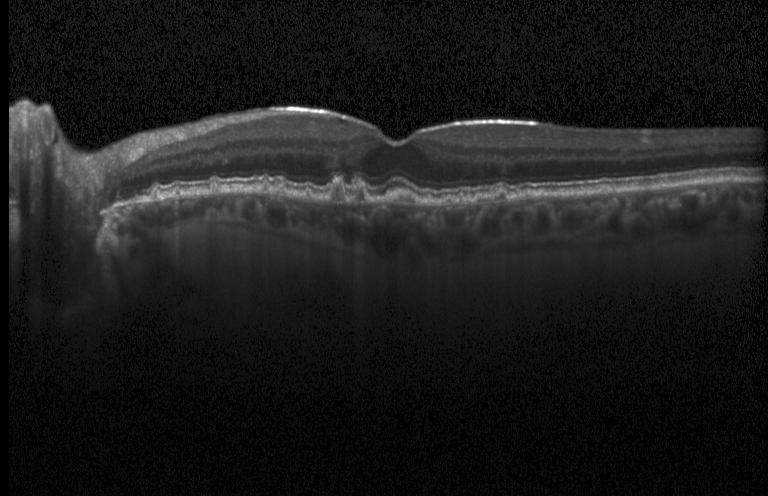 Impression: sub-RPE drusenoid deposits.